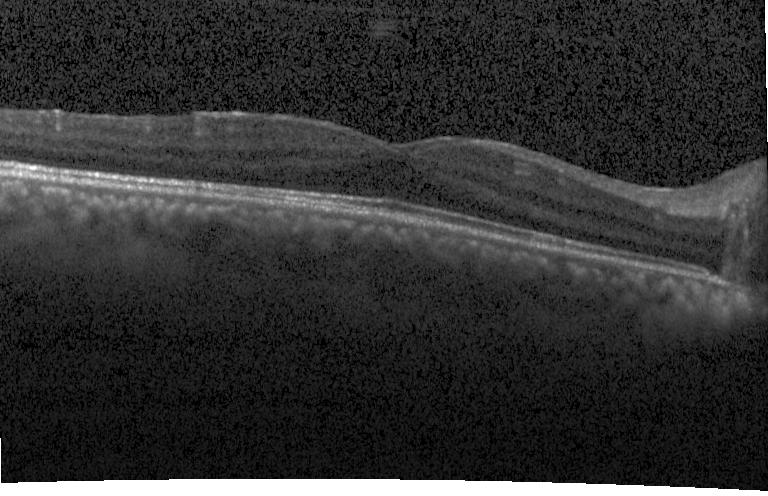

Retinal OCT cross-section showing no evidence of choroidal neovascularization, diabetic macular edema, or drusen.